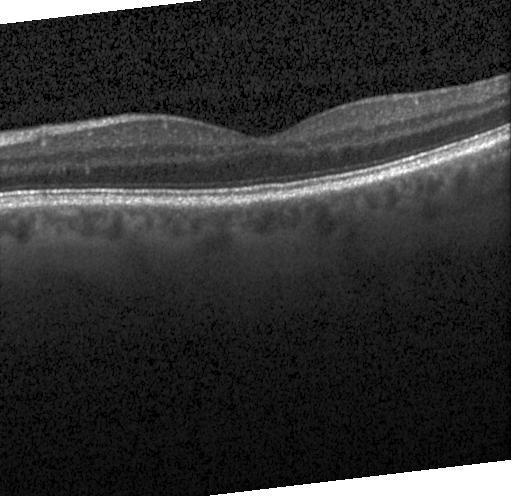
Retinal OCT B-scan. Acquired on a Heidelberg Spectralis — Dx: no choroidal neovascularization, no diabetic macular edema, and no drusen.